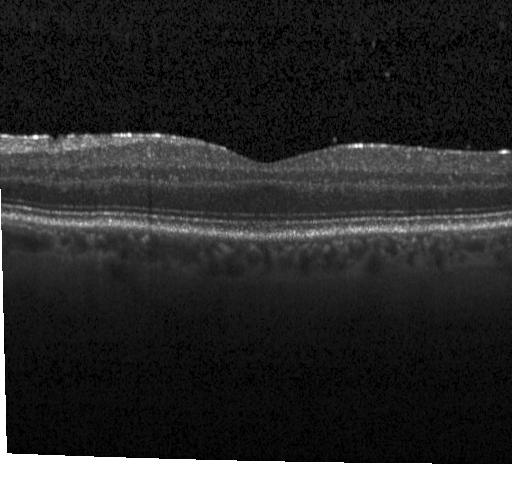
Optical coherence tomography scan
Macular OCT: no evidence of choroidal neovascularization, diabetic macular edema, or drusen.